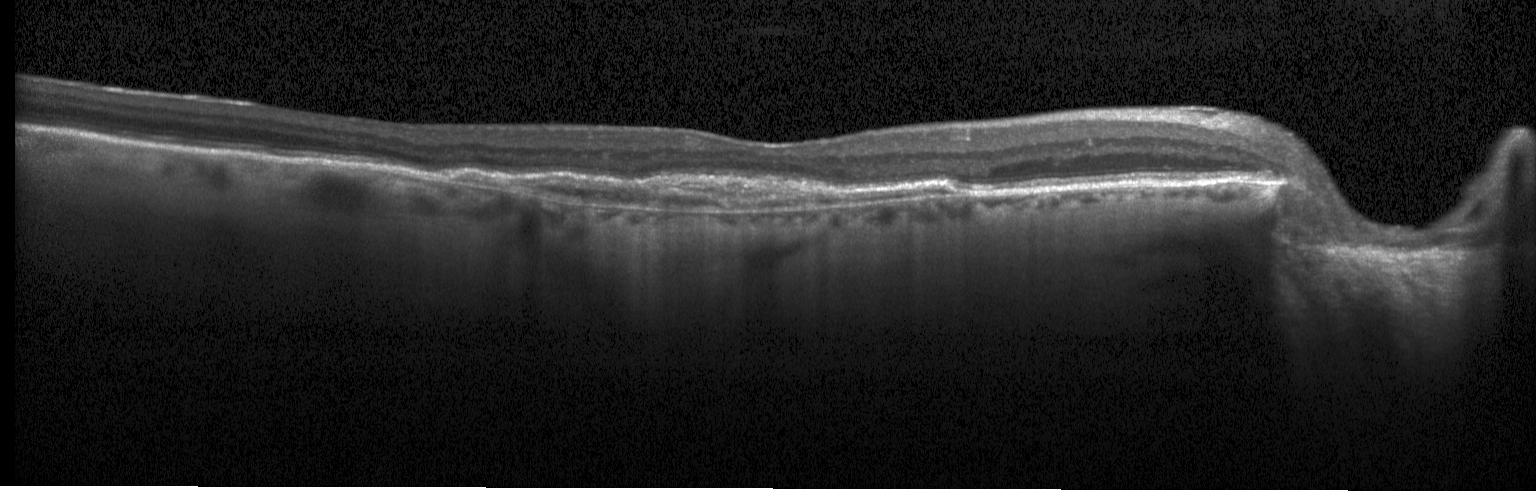
Optical coherence tomography B-scan. Acquired on a Heidelberg Spectralis. OCT finding: a choroidal neovascular membrane.